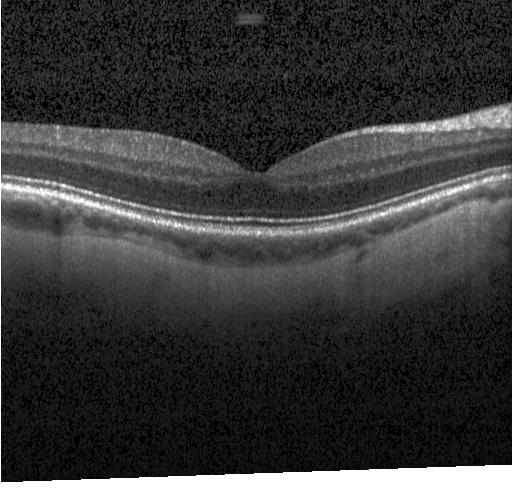
Fovea-centered. Spectral-domain optical coherence tomography. Acquired on a Heidelberg Spectralis. Retinal OCT B-scan.
Impression: no evidence of choroidal neovascularization, diabetic macular edema, or drusen.